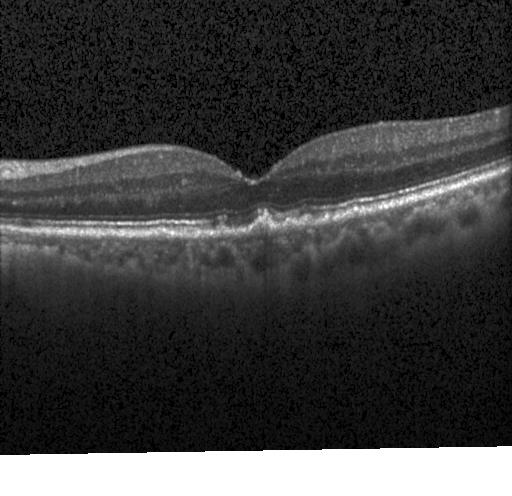 Impression: drusen.